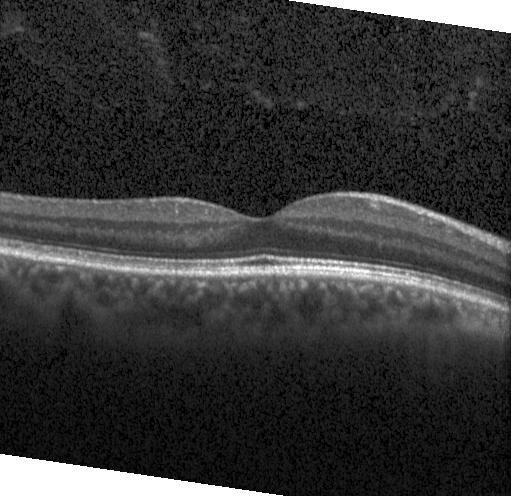

Diagnosis: no choroidal neovascularization, no diabetic macular edema, and no drusen.